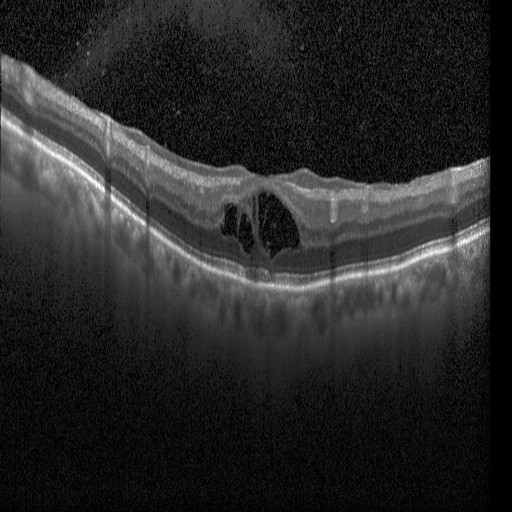

Retinal OCT cross-section showing diabetic macular edema (DME).